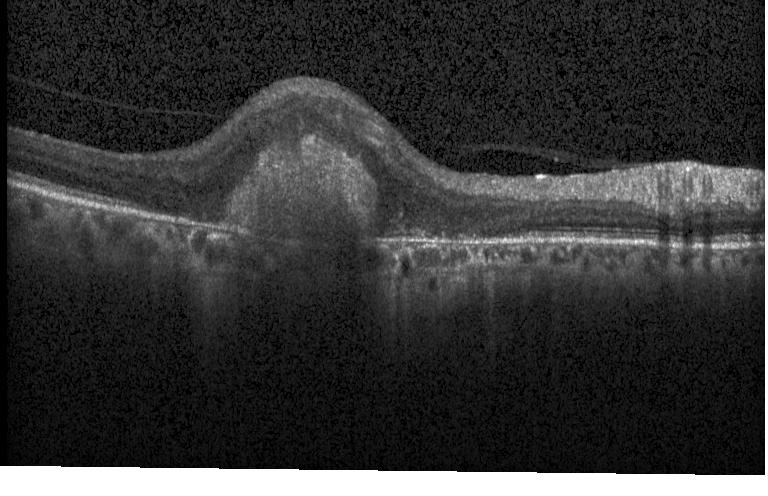

Finding: a choroidal neovascular membrane.